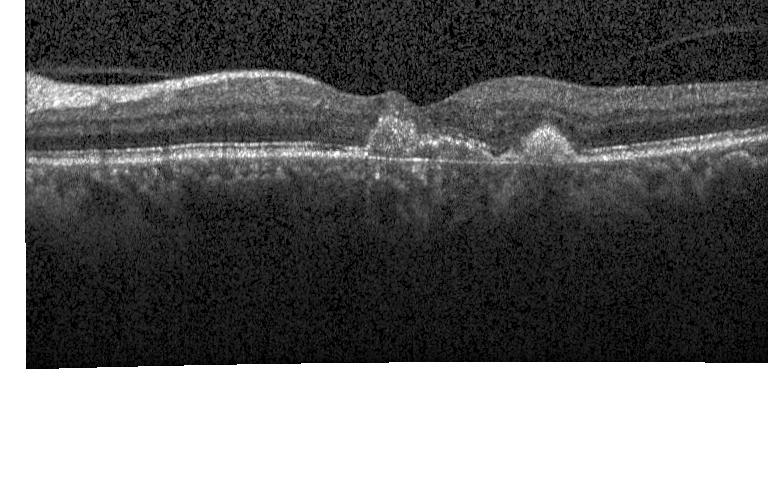 Retinal OCT cross-section, horizontal scan through the fovea, acquired on a Heidelberg Spectralis, spectral-domain optical coherence tomography. Finding: a choroidal neovascular membrane.